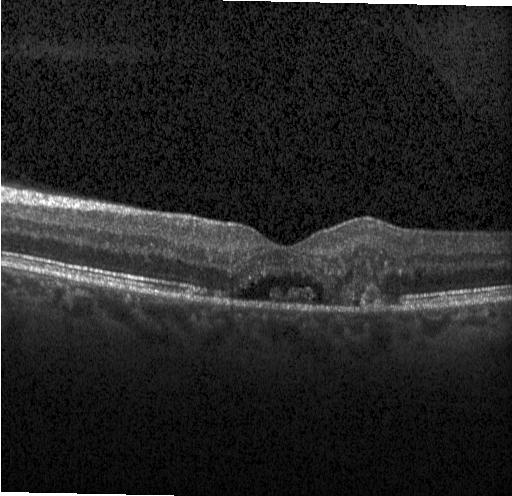

Diagnosis: choroidal neovascularization.